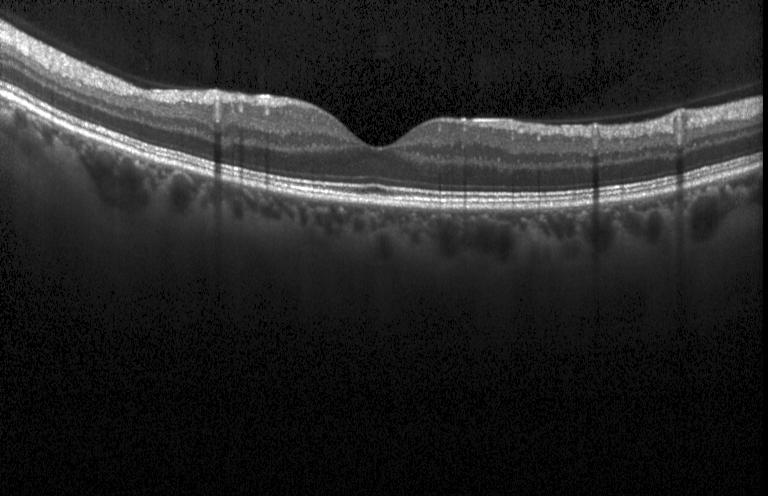 Retinal OCT cross-section showing no choroidal neovascularization, diabetic macular edema, or drusen.